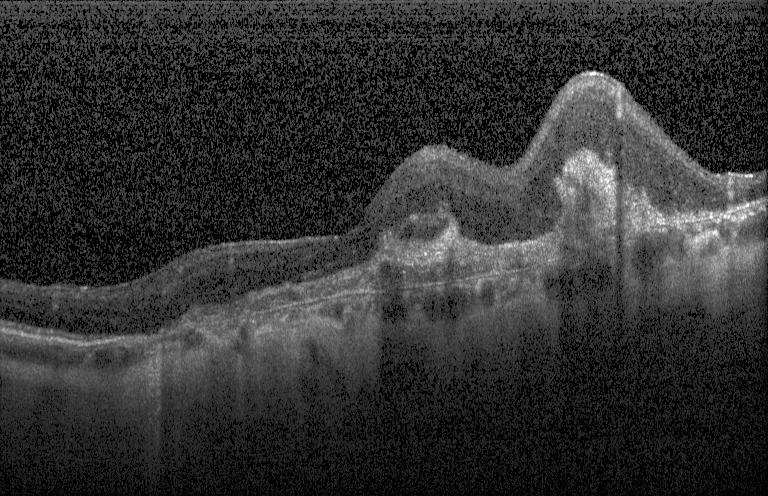
Heidelberg Spectralis OCT system, SD-OCT, retinal OCT B-scan — The scan shows a choroidal neovascular membrane.